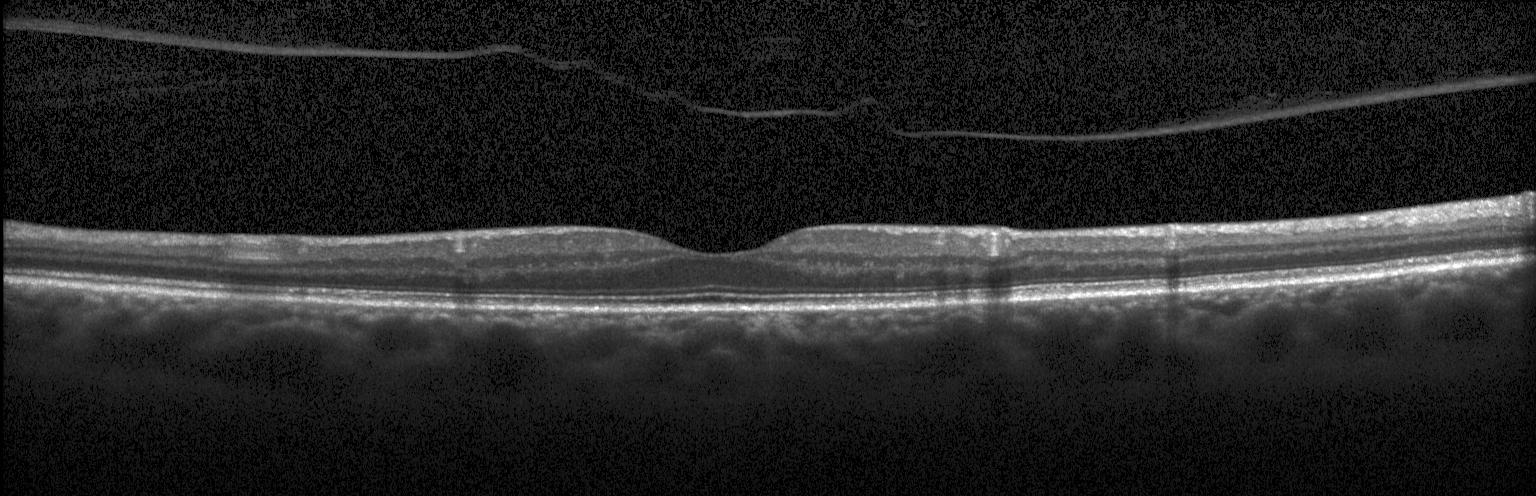

Retinal OCT B-scan, spectral-domain optical coherence tomography — Impression: neither choroidal neovascularization, diabetic macular edema, nor drusen.